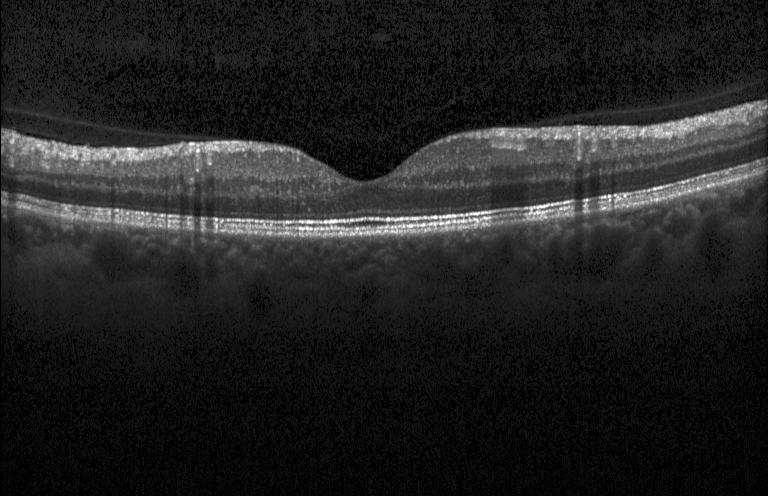 Assessment: no choroidal neovascularization, diabetic macular edema, or drusen.